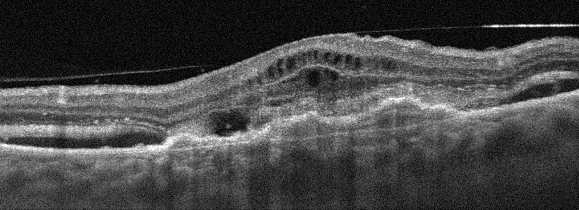
Retinal OCT cross-section. Left eye — Impression: age-related macular degeneration.